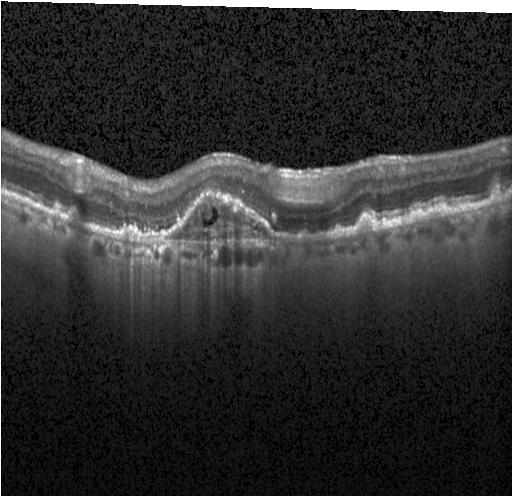 Spectral-domain OCT B-scan: a choroidal neovascular membrane.